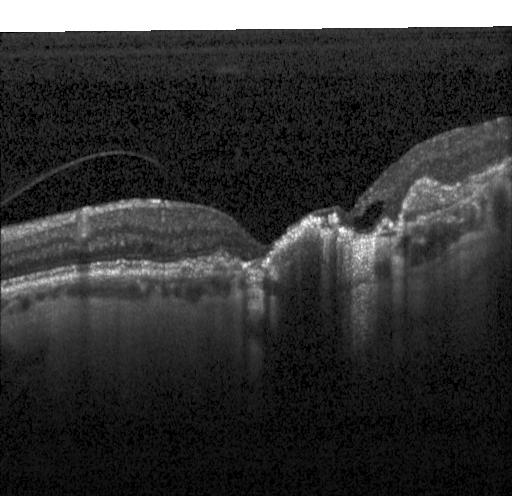
Macular OCT demonstrating choroidal neovascularization (CNV).